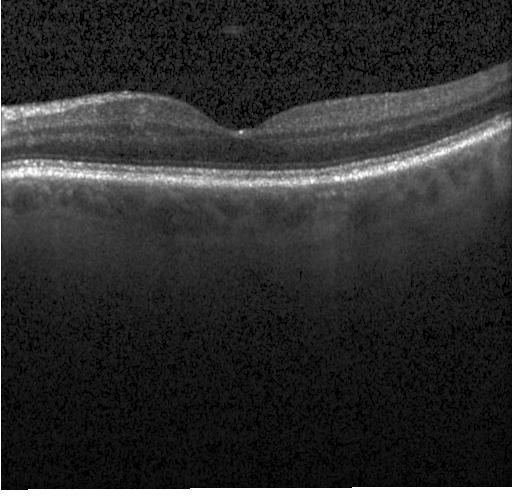

Impression: no evidence of CNV, DME, or drusen.